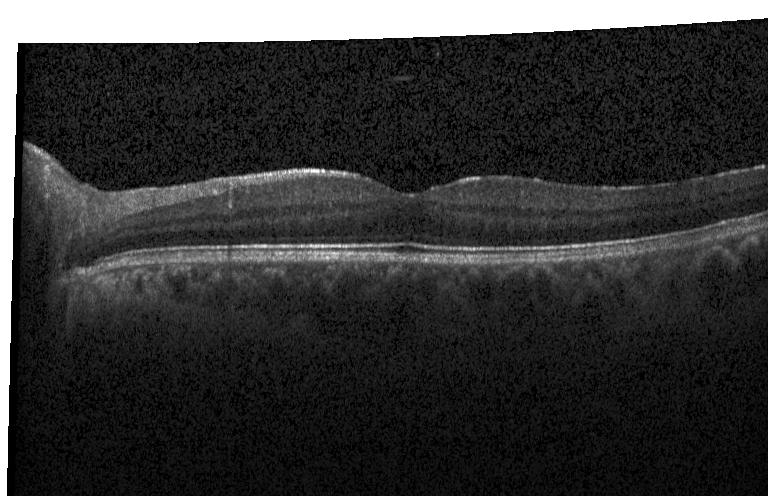 Horizontal scan through the fovea; SD-OCT; OCT B-scan — Diagnosis: neither CNV, DME, nor drusen.